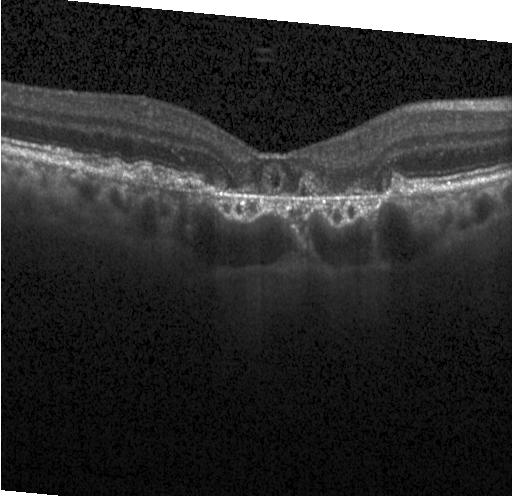

Heidelberg Spectralis · OCT B-scan · horizontal scan through the fovea · spectral-domain OCT
The scan shows choroidal neovascularization (CNV).